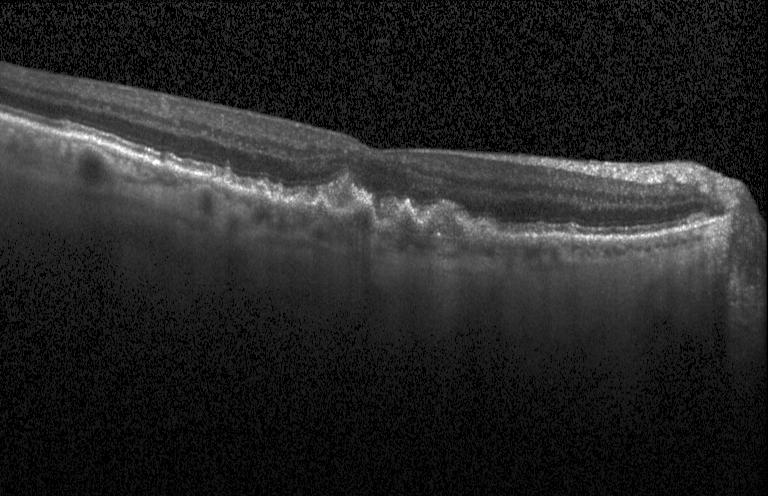 Macular OCT demonstrating a choroidal neovascular membrane.